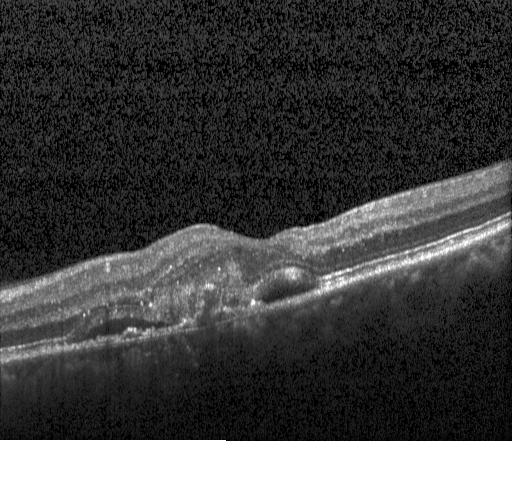
Optical coherence tomography B-scan. Fovea-centered. Spectral-domain optical coherence tomography.
This B-scan demonstrates a choroidal neovascular membrane.